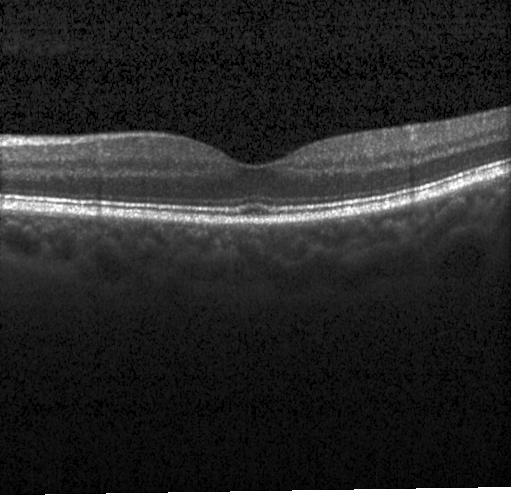
OCT line scan
Impression: no CNV, DME, or drusen.